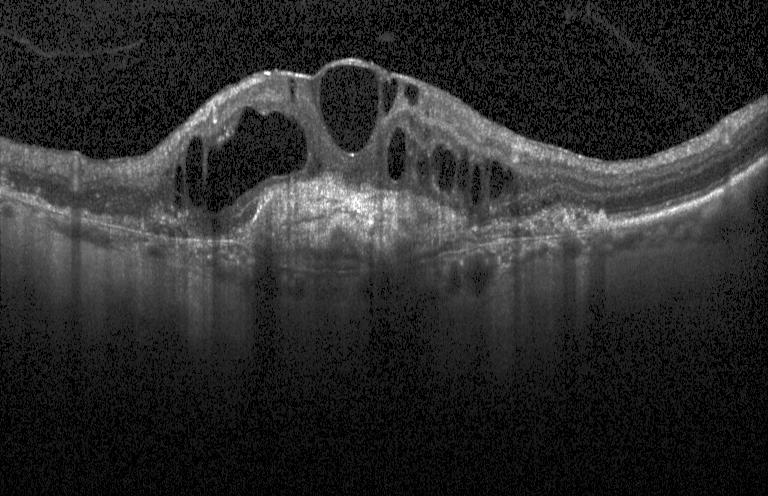 Impression: a choroidal neovascular membrane.